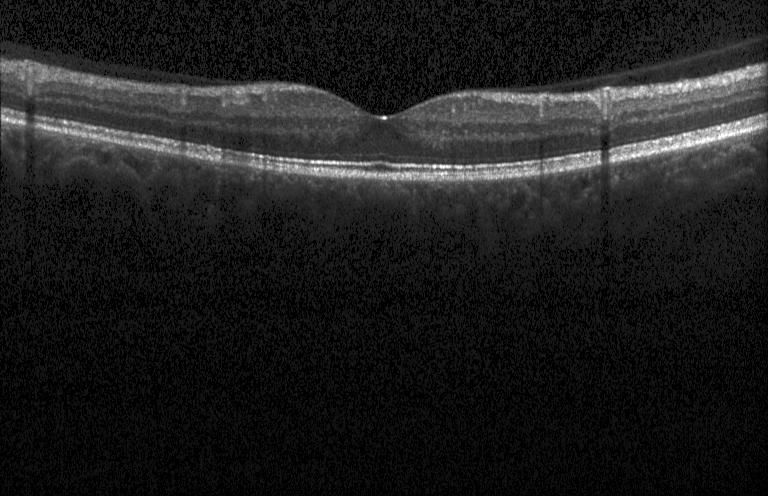
SD-OCT. OCT line scan. Heidelberg Spectralis — The scan shows no CNV, DME, or drusen.